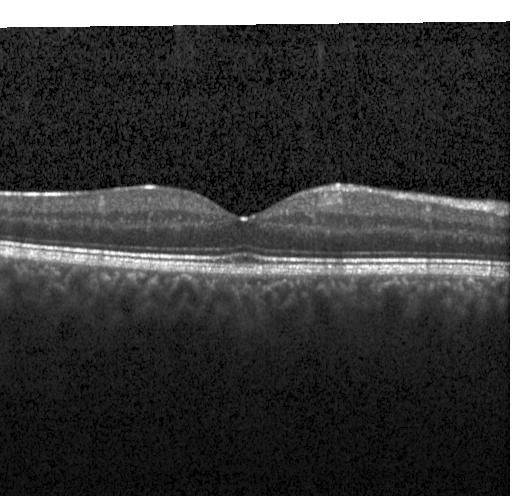 Retinal OCT cross-section showing neither CNV, DME, nor drusen.